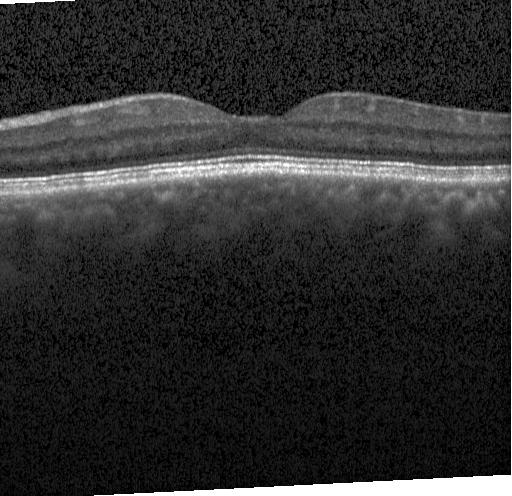

Retinal OCT cross-section showing no evidence of CNV, DME, or drusen.